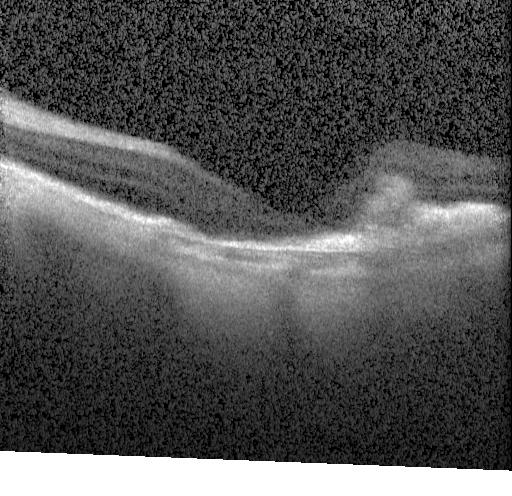
OCT scan showing choroidal neovascularization.